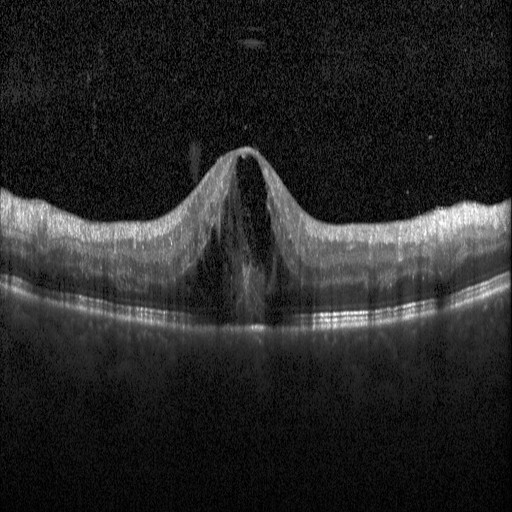

Finding: diabetic macular edema.